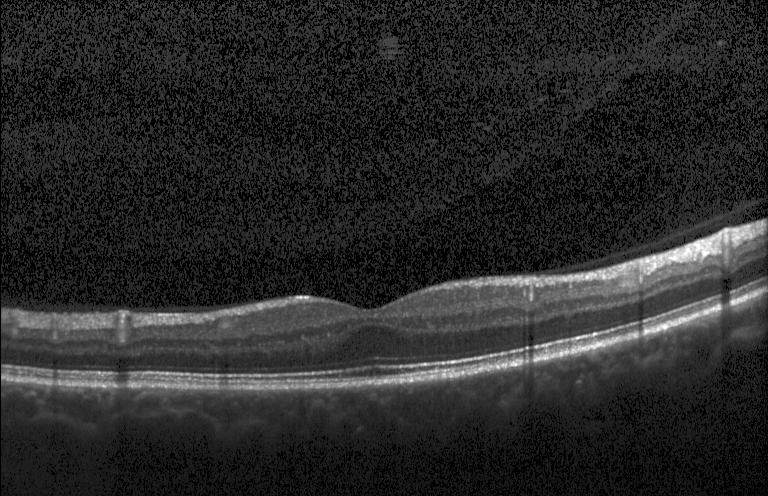

Finding: neither choroidal neovascularization, diabetic macular edema, nor drusen.